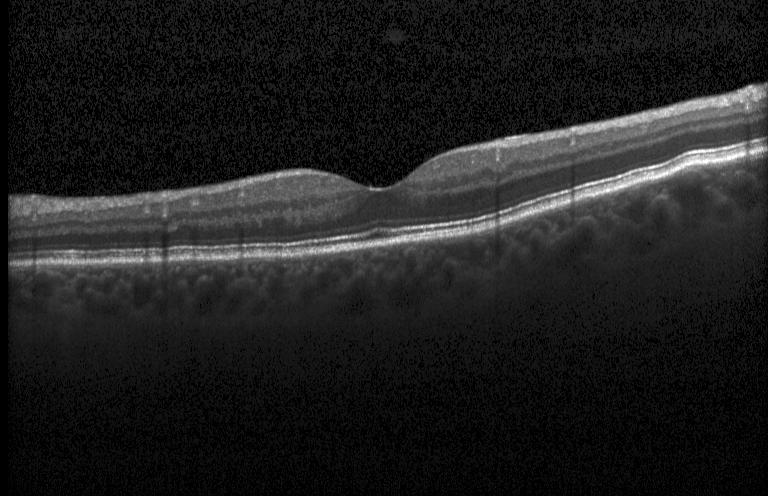
Heidelberg Spectralis OCT system, optical coherence tomography scan, spectral-domain optical coherence tomography — Macular OCT: no choroidal neovascularization, no diabetic macular edema, and no drusen.